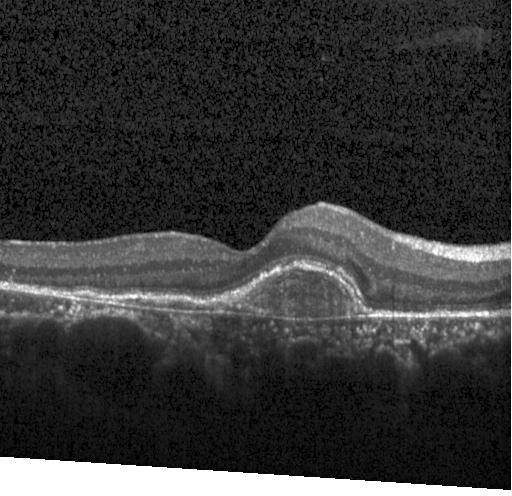
Spectral-domain optical coherence tomography, OCT line scan. Finding: a choroidal neovascular membrane.